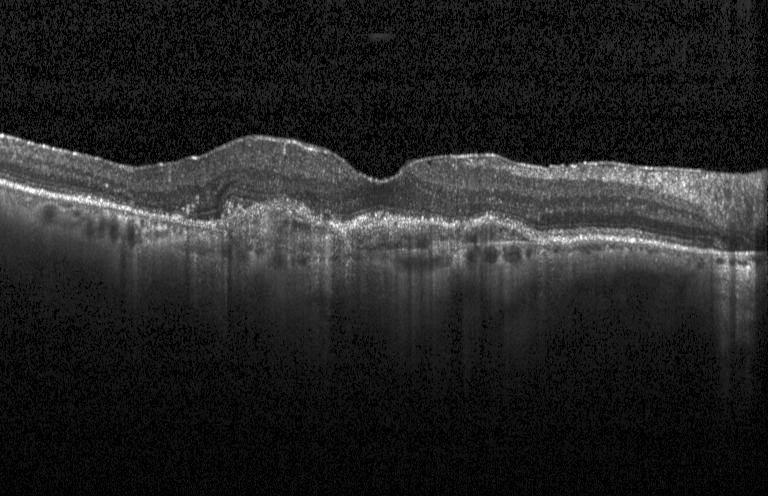
Heidelberg Spectralis · horizontal scan through the fovea · OCT line scan · spectral-domain OCT.
Impression: a choroidal neovascular membrane.